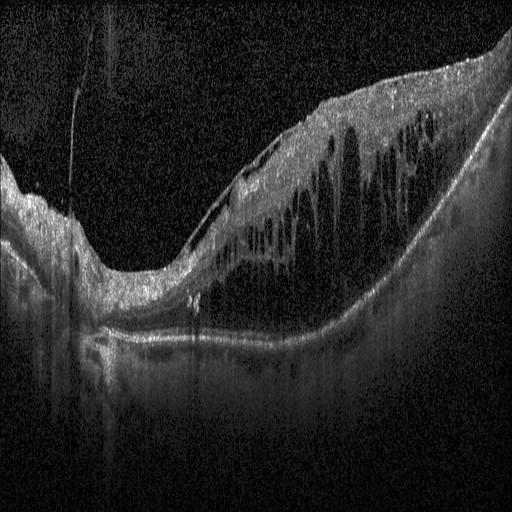
Instrument: Heidelberg Spectralis; OCT line scan. Diagnosis: diabetic macular edema.